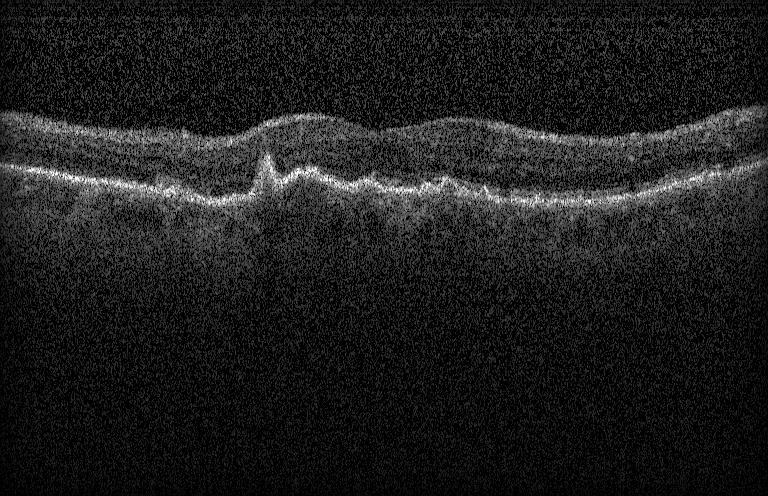

Macular scan, retinal OCT cross-section. Diagnosis: a choroidal neovascular membrane.